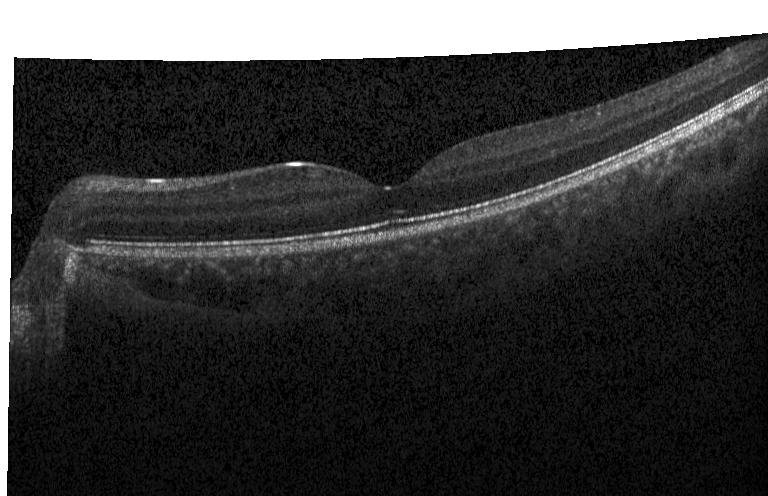
Diagnosis: neither CNV, DME, nor drusen.